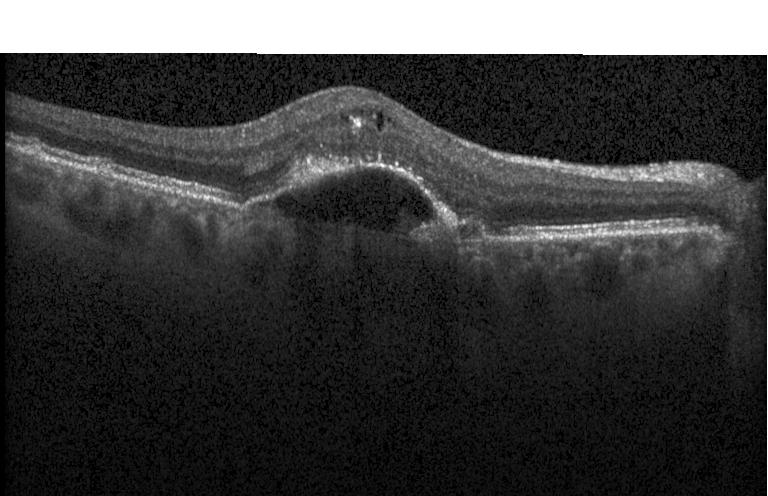

Finding: a choroidal neovascular membrane.